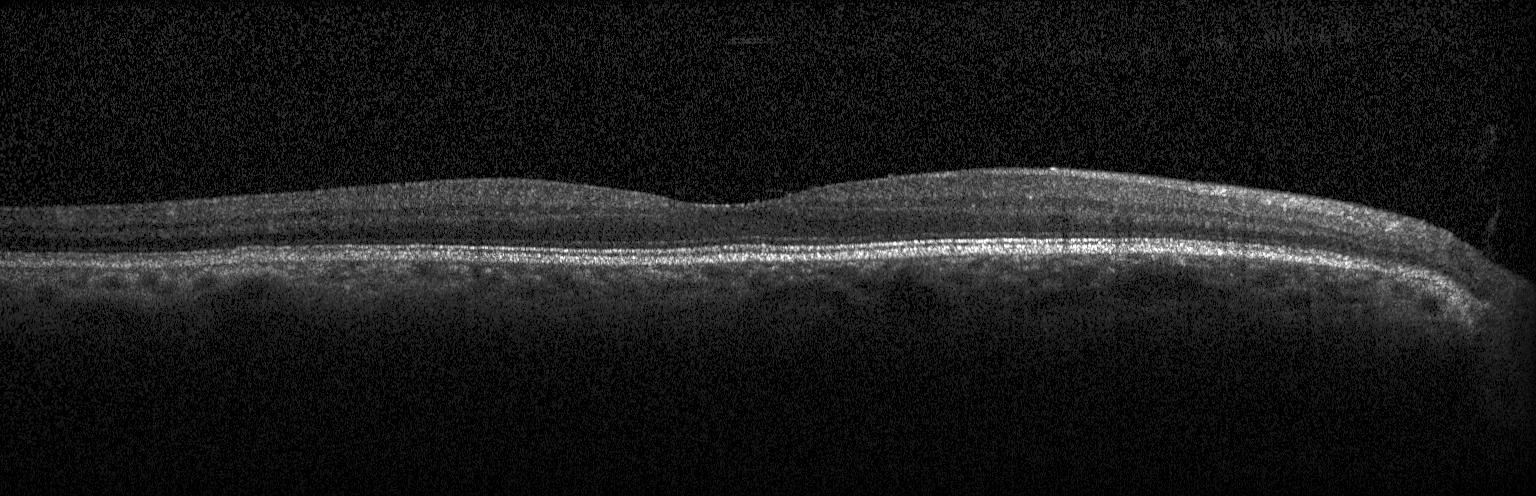

Macular OCT demonstrating no evidence of choroidal neovascularization, diabetic macular edema, or drusen.